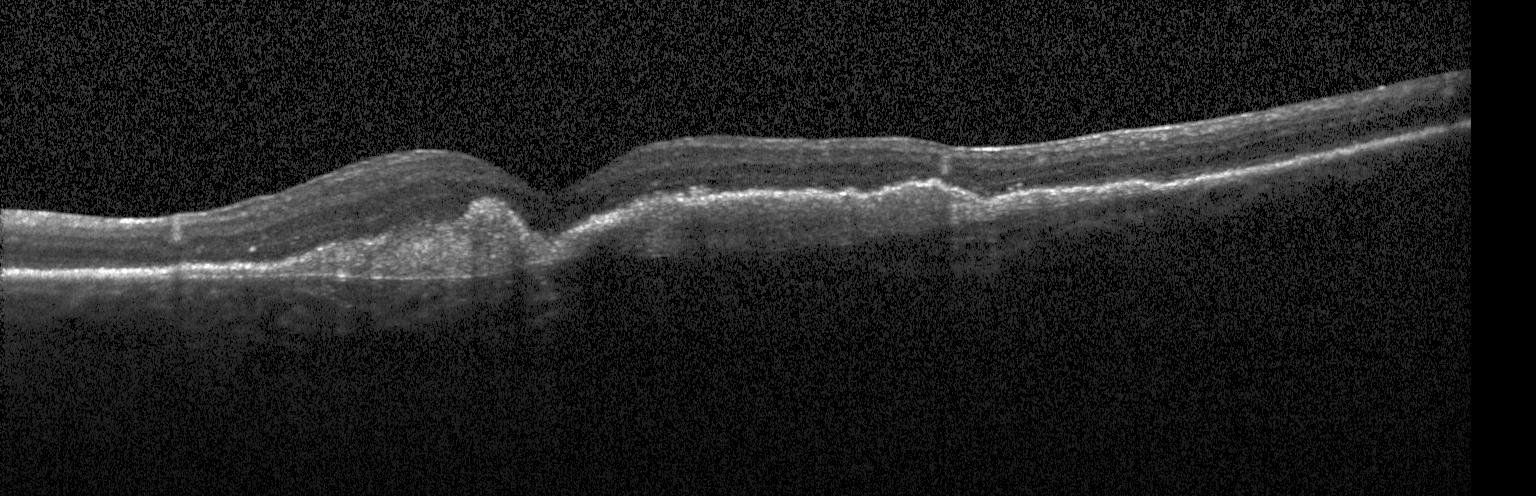
OCT line scan · SD-OCT · Heidelberg Spectralis · fovea-centered
Choroidal neovascularization (CNV).